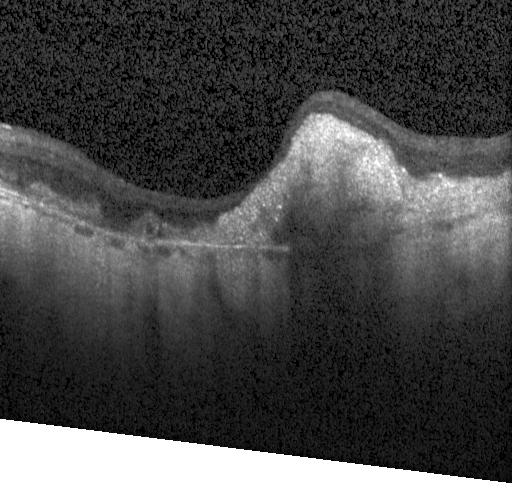

Optical coherence tomography B-scan — Impression: a choroidal neovascular membrane.